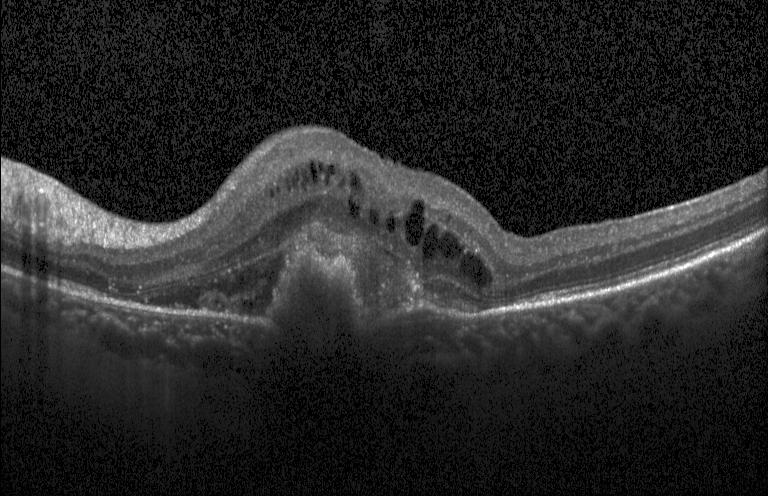

Optical coherence tomography scan; Heidelberg Spectralis OCT system. Diagnosis: choroidal neovascularization.